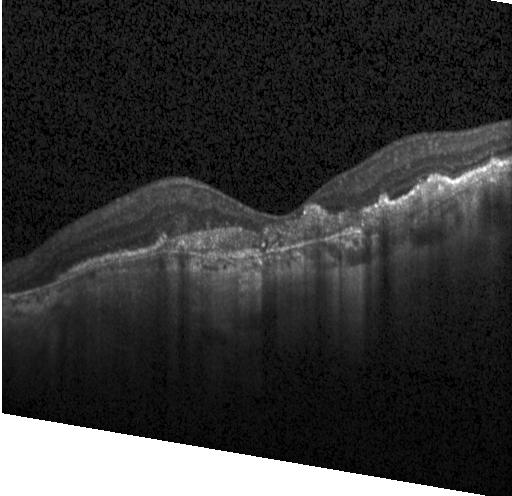
Acquired on a Heidelberg Spectralis; retinal OCT B-scan.
Impression: choroidal neovascularization (CNV).